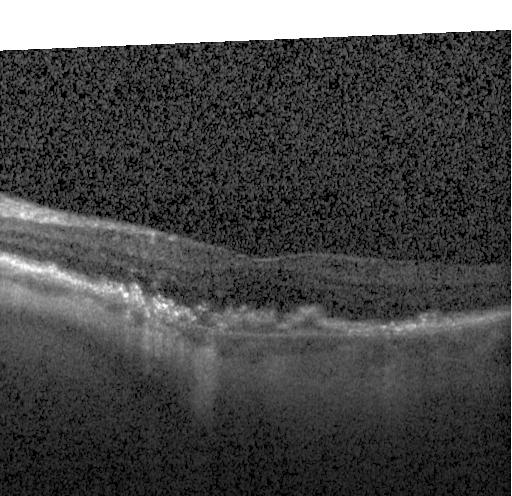

Heidelberg Spectralis, centered on the fovea, OCT line scan. Diagnosis: choroidal neovascularization.